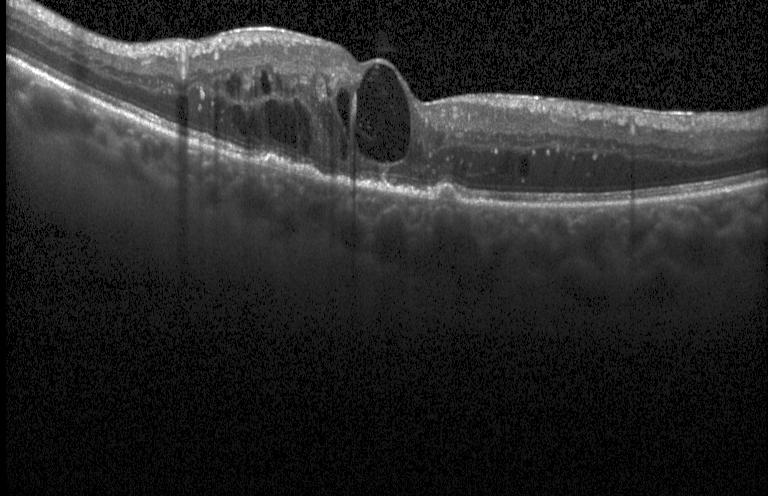
Assessment: diabetic macular edema.